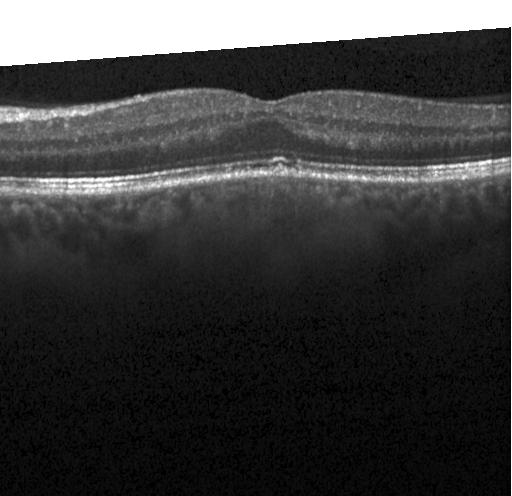
Optical coherence tomography scan; acquired on a Heidelberg Spectralis; horizontal scan through the fovea — Finding: no evidence of choroidal neovascularization, diabetic macular edema, or drusen.